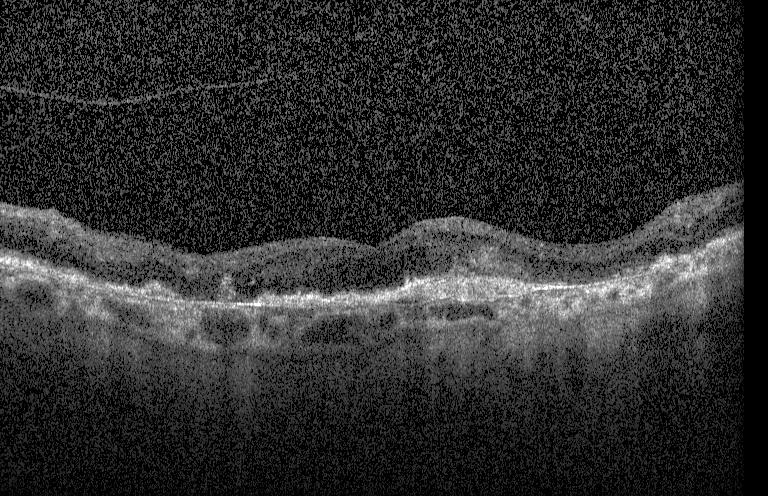
Finding: CNV.